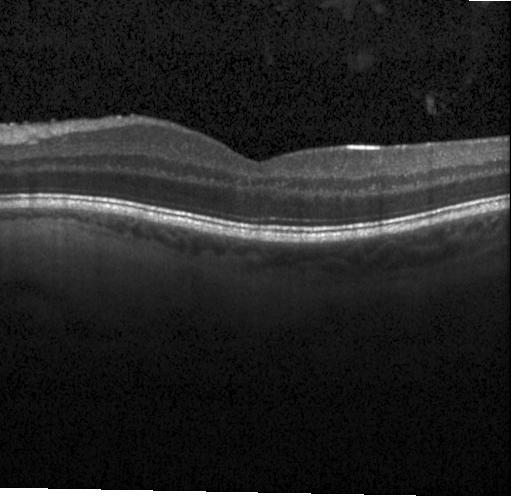
Heidelberg Spectralis; OCT line scan.
The scan shows neither choroidal neovascularization, diabetic macular edema, nor drusen.